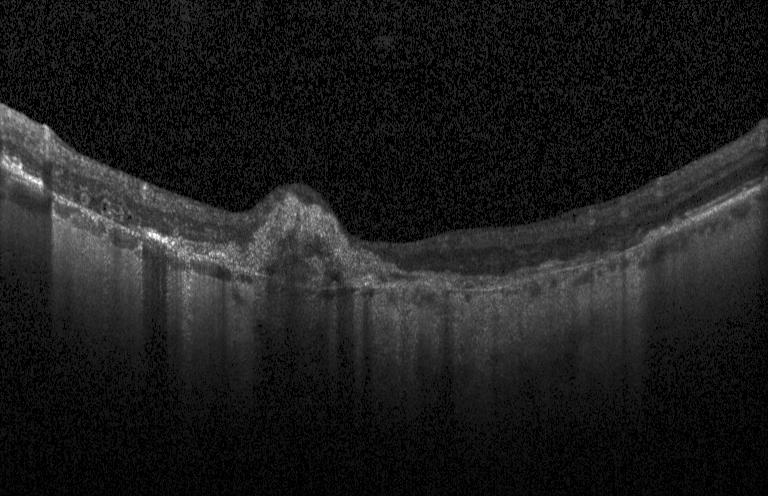
Optical coherence tomography scan, spectral-domain OCT, fovea-centered. Diagnosis: a choroidal neovascular membrane.